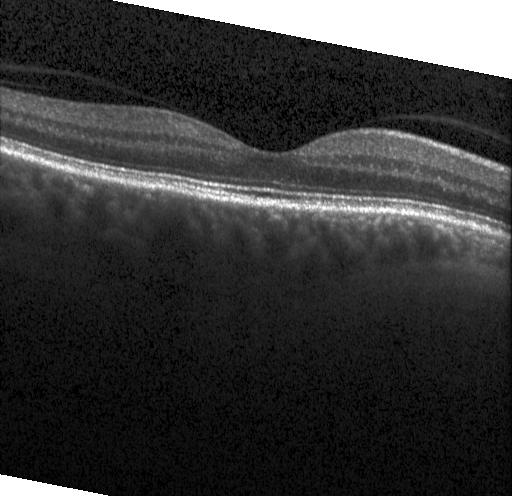

Retinal OCT cross-section showing no choroidal neovascularization, diabetic macular edema, or drusen.